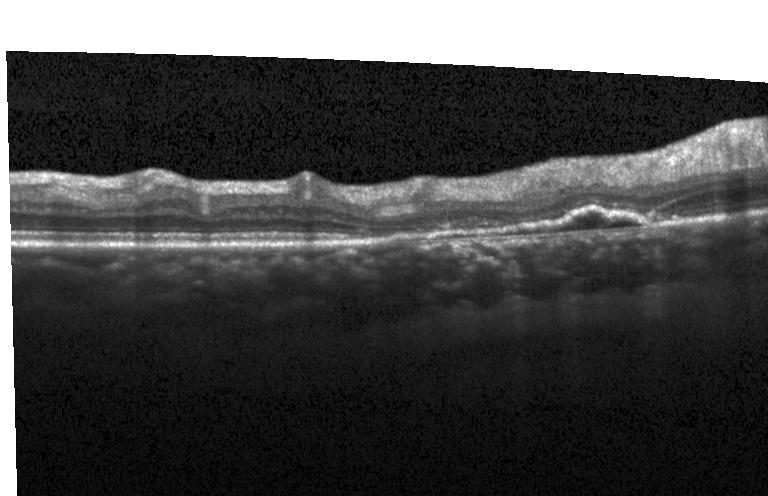

OCT B-scan showing a choroidal neovascular membrane.